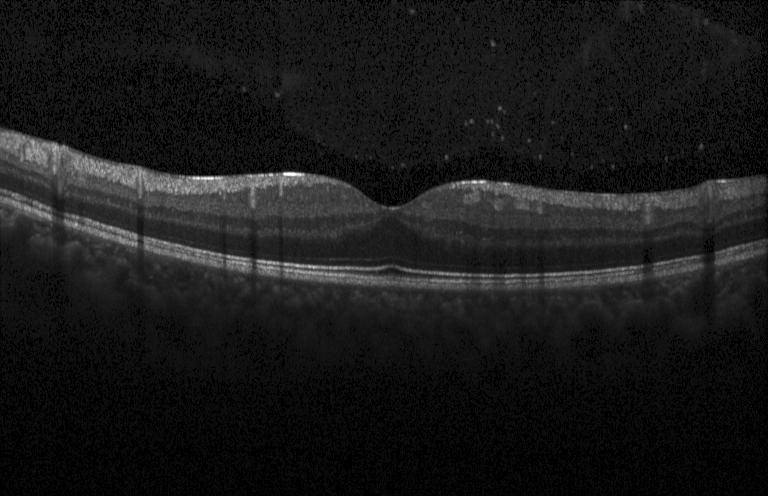

Diagnosis: no CNV, DME, or drusen.